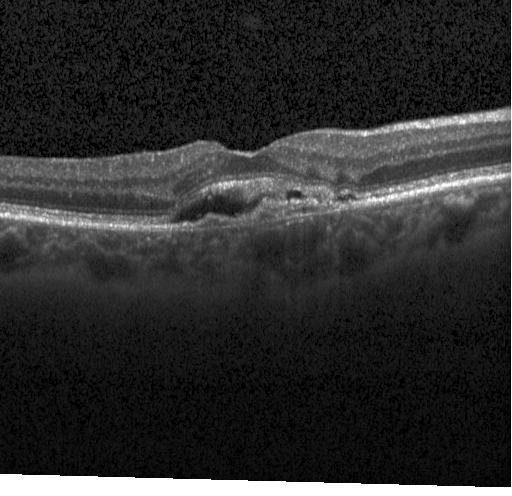
The scan shows a choroidal neovascular membrane.